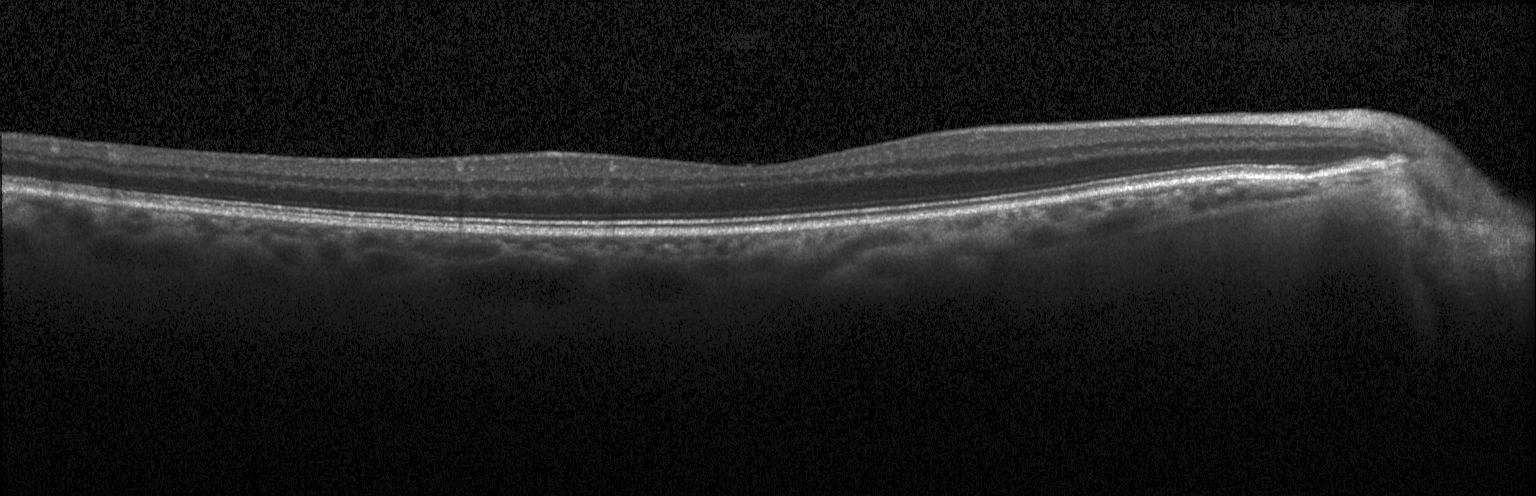

Retinal OCT cross-section — Diagnosis: no choroidal neovascularization, no diabetic macular edema, and no drusen.